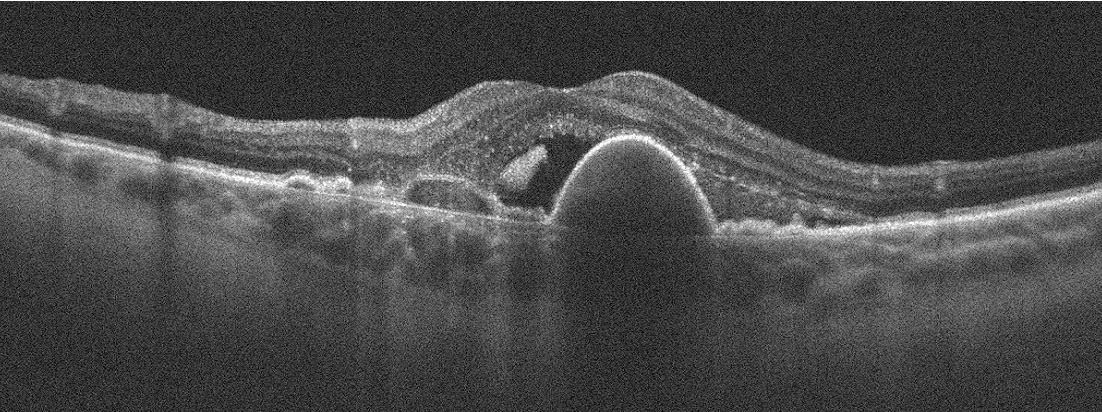 Dx: AMD.